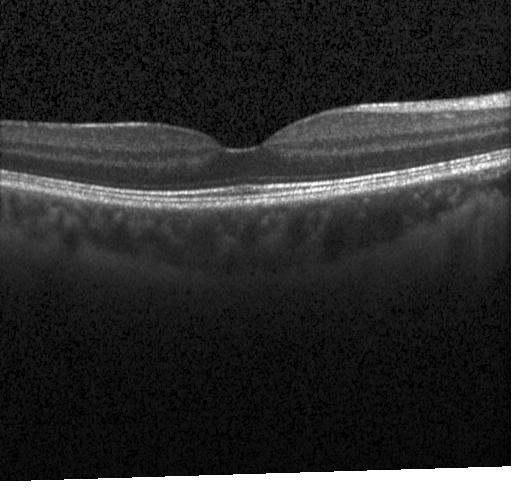
OCT B-scan. Instrument: Heidelberg Spectralis
No choroidal neovascularization, no diabetic macular edema, and no drusen.